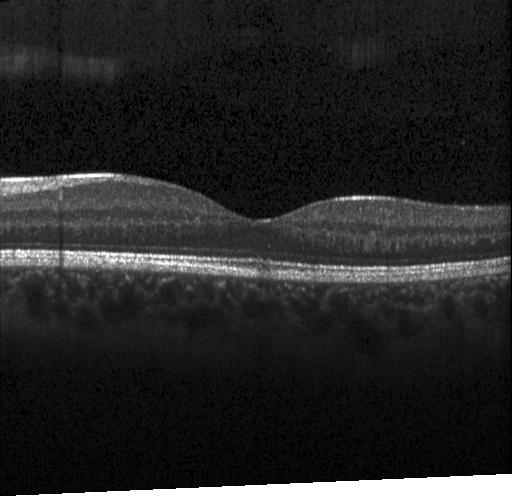
Assessment: neither choroidal neovascularization, diabetic macular edema, nor drusen.